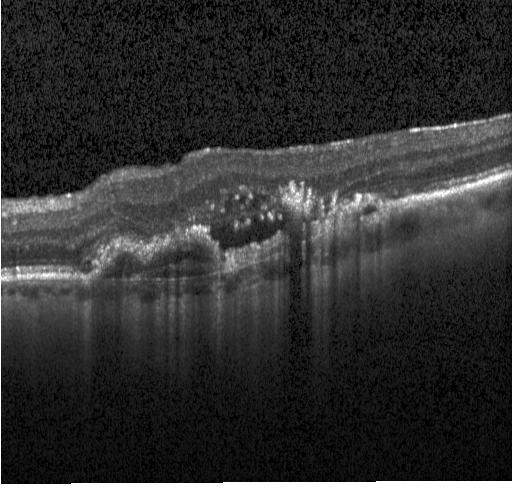 Macular OCT demonstrating CNV.